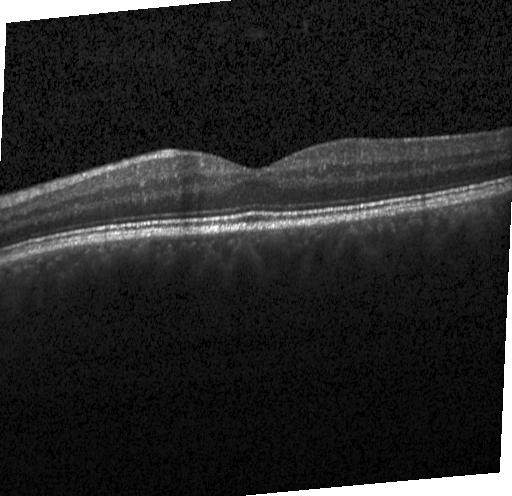 Centered on the fovea, OCT line scan, SD-OCT.
Finding: no CNV, DME, or drusen.